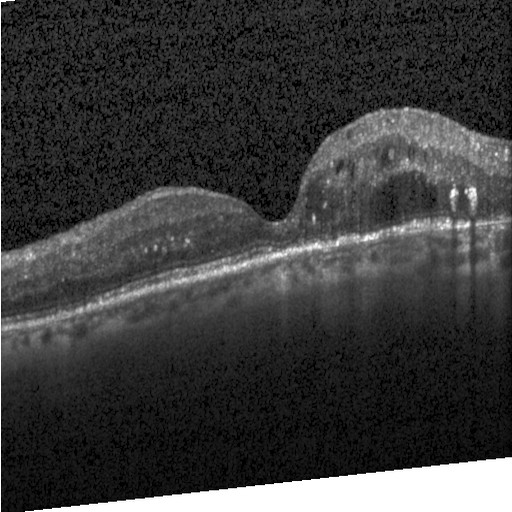 Retinal OCT B-scan. Heidelberg Spectralis. Horizontal scan through the fovea. Spectral-domain optical coherence tomography
Impression: diabetic macular edema (DME).